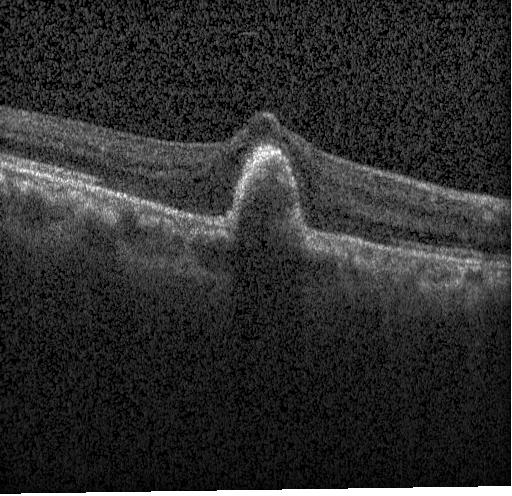

Retinal OCT B-scan
Diagnosis: a choroidal neovascular membrane.